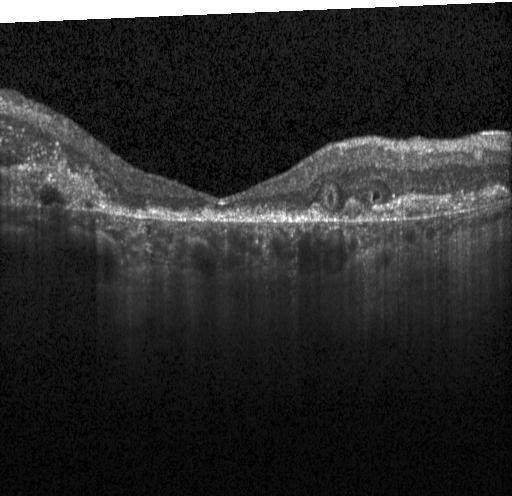
OCT B-scan; horizontal scan through the fovea; spectral-domain optical coherence tomography; Heidelberg Spectralis. Finding: CNV.